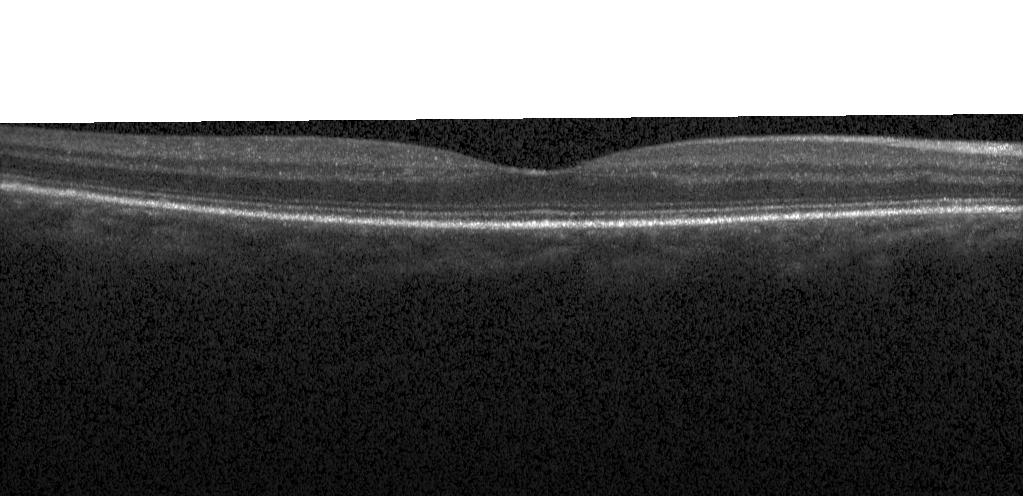

Retinal OCT cross-section showing no evidence of choroidal neovascularization, diabetic macular edema, or drusen.